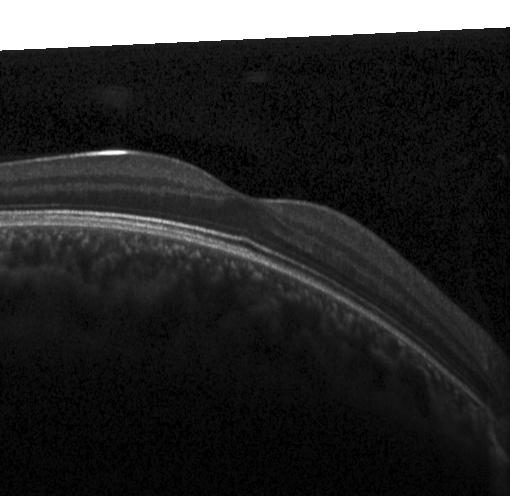

Dx: no CNV, no DME, and no drusen.